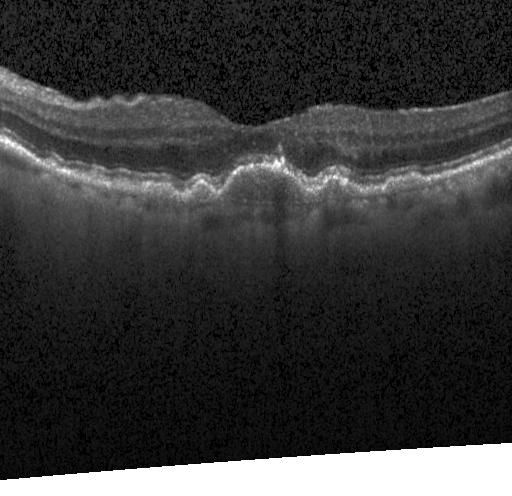 Retinal OCT B-scan · SD-OCT · through the macula · acquired on a Heidelberg Spectralis — Diagnosis: a choroidal neovascular membrane.